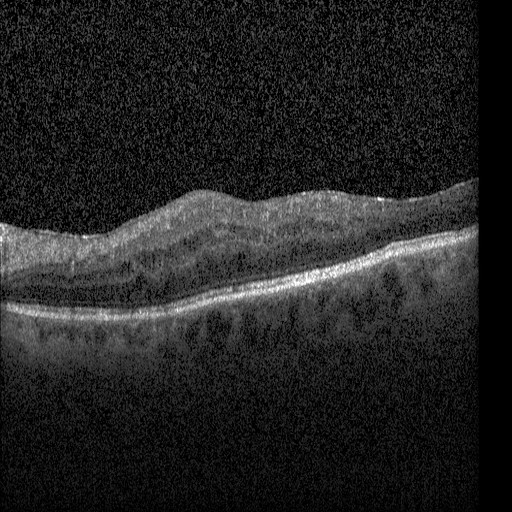 OCT scan showing diabetic macular edema (DME).